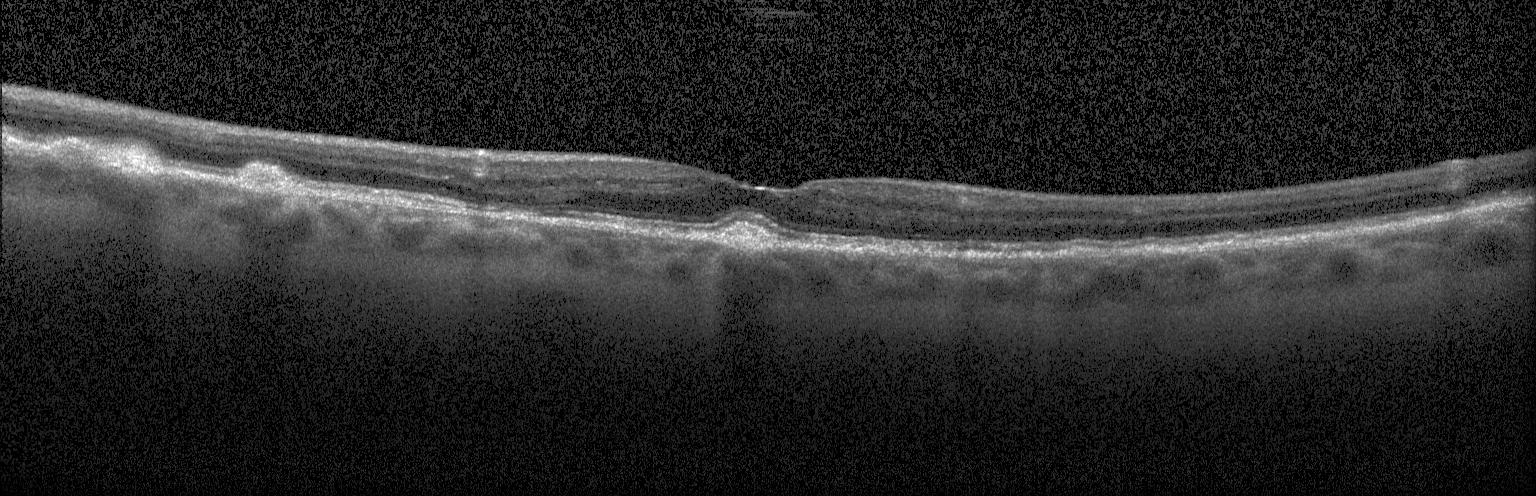
Retinal OCT cross-section showing sub-RPE drusenoid deposits.